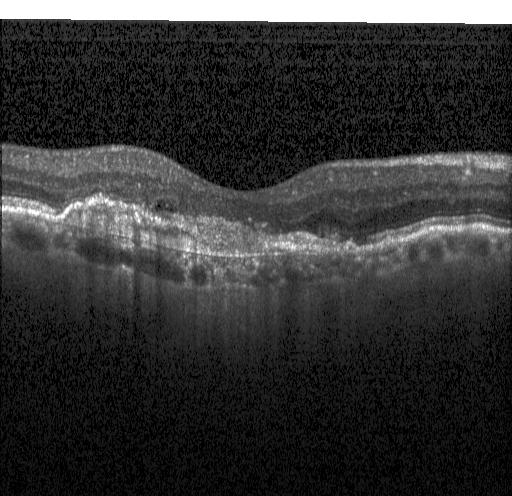 Heidelberg Spectralis, SD-OCT, through the macula, optical coherence tomography scan
A choroidal neovascular membrane.